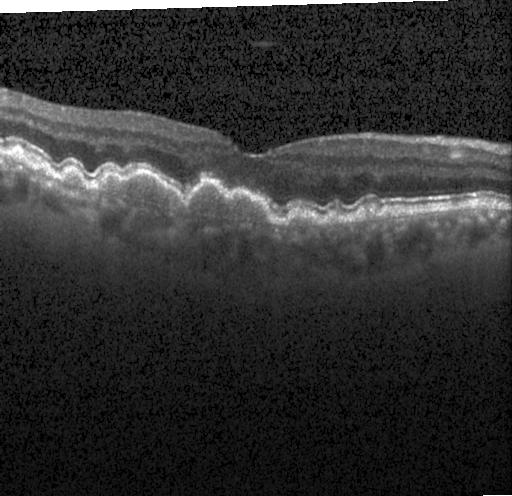
Impression: multiple drusen.